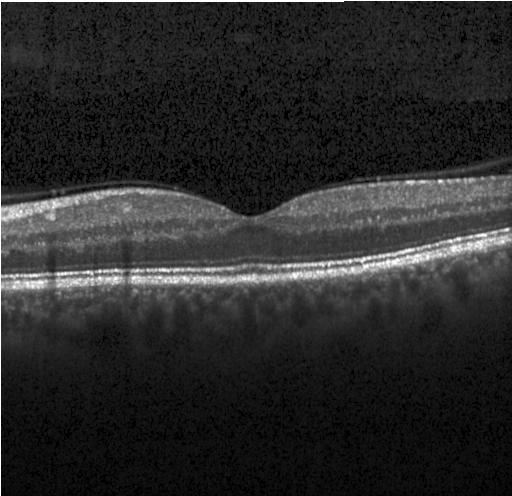

Retinal OCT B-scan, SD-OCT. No evidence of choroidal neovascularization, diabetic macular edema, or drusen.